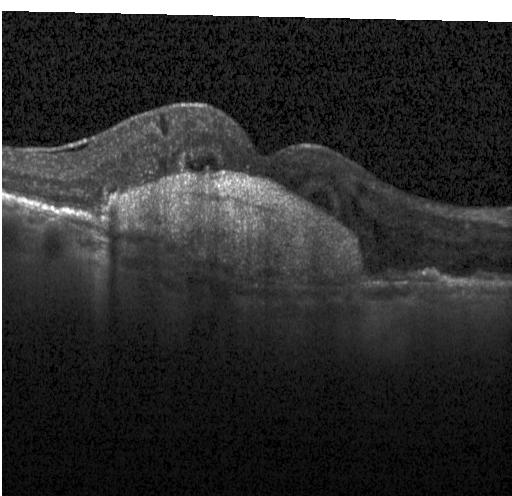
Centered on the fovea. Optical coherence tomography B-scan — Finding: choroidal neovascularization (CNV).